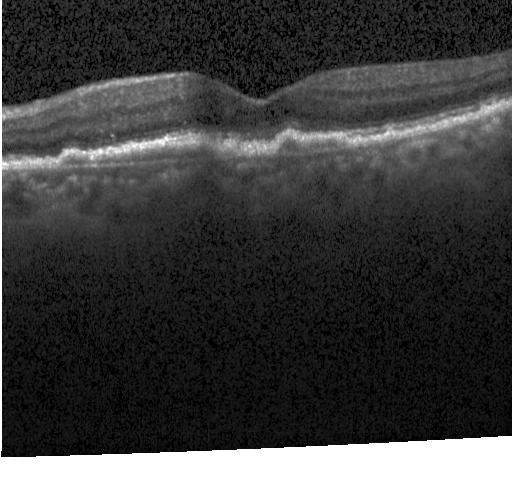

OCT finding: a choroidal neovascular membrane.